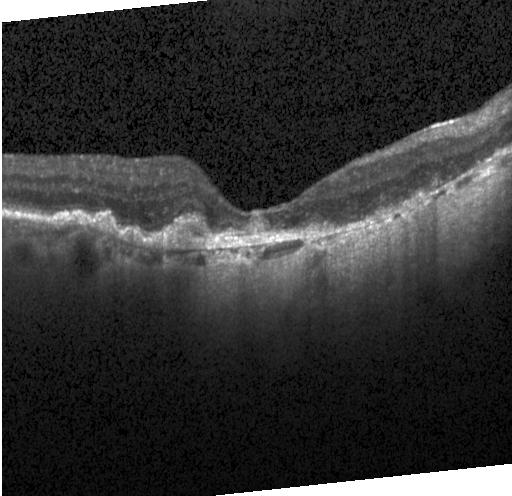 OCT line scan
CNV.